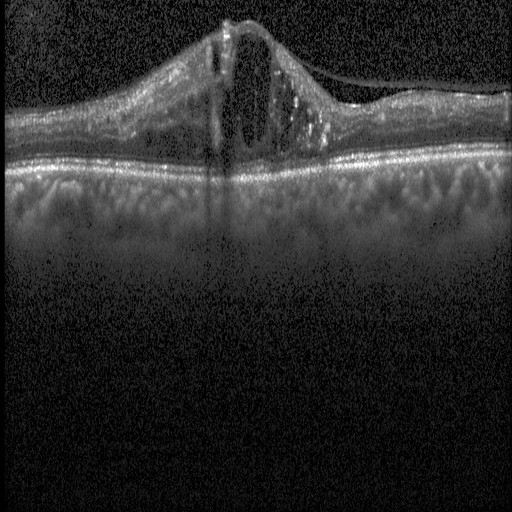
Impression: diabetic macular edema (DME).